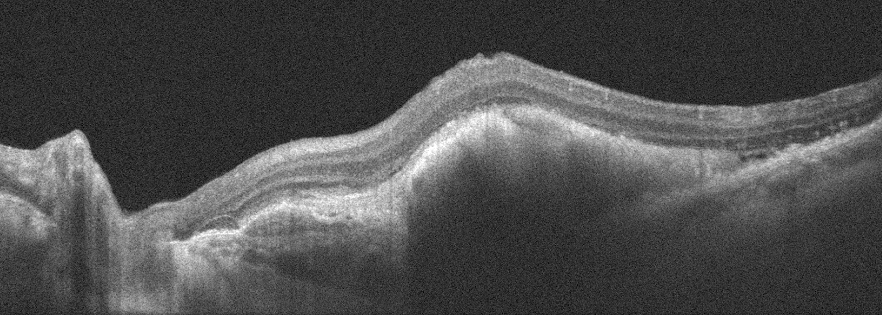
Oculus sinister · retinal OCT B-scan · through the macula.
Finding: age-related macular degeneration (AMD).